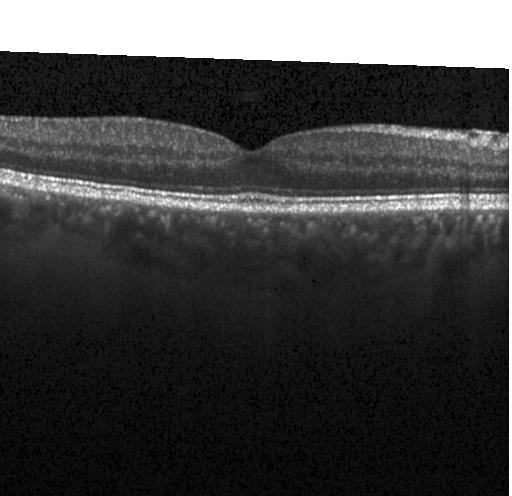 Spectral-domain OCT B-scan: no CNV, no DME, and no drusen.